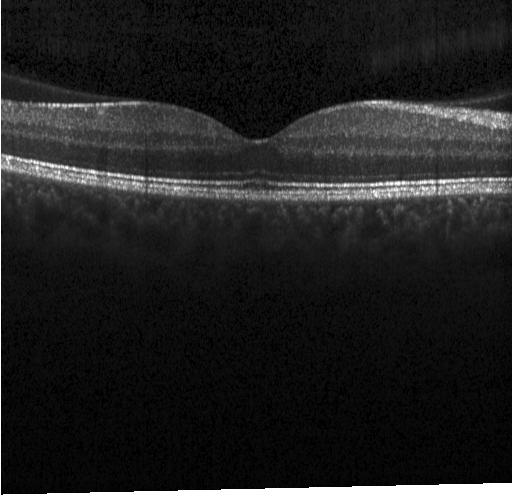
Heidelberg Spectralis OCT system. Optical coherence tomography B-scan. Finding: no evidence of choroidal neovascularization, diabetic macular edema, or drusen.